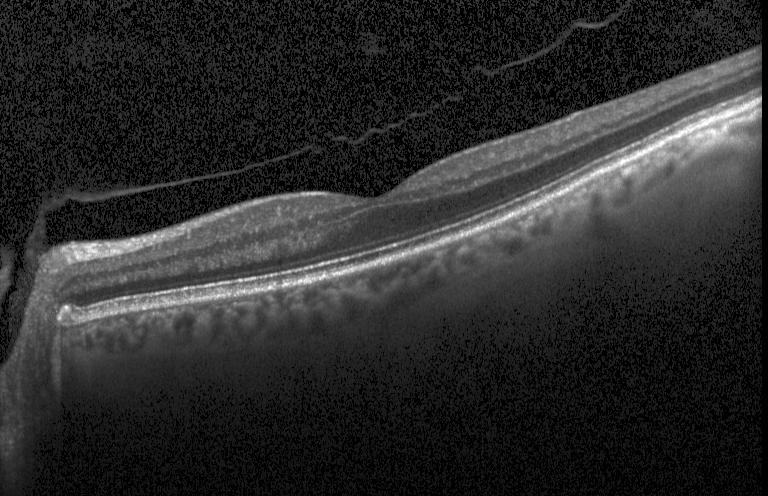
Fovea-centered · optical coherence tomography scan · spectral-domain OCT.
Assessment: neither choroidal neovascularization, diabetic macular edema, nor drusen.